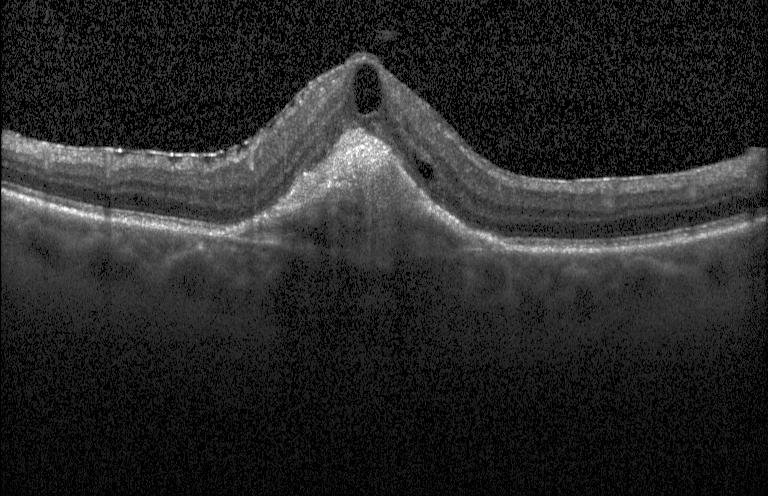

Retinal OCT B-scan — Macular OCT: choroidal neovascularization.